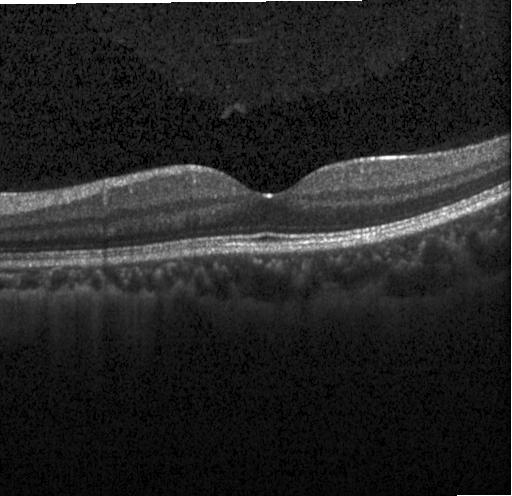

Macular OCT: neither choroidal neovascularization, diabetic macular edema, nor drusen.